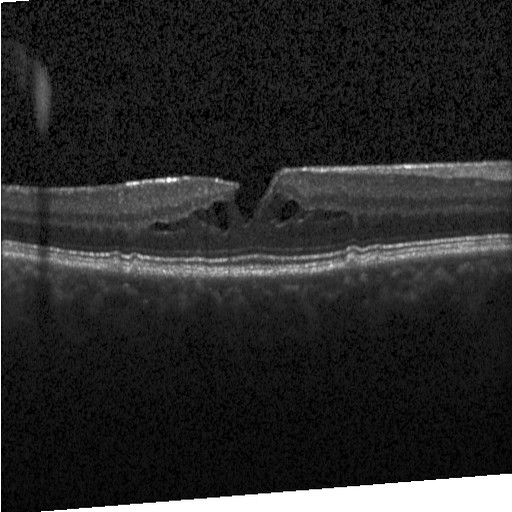
Diagnosis: diabetic macular edema (DME).